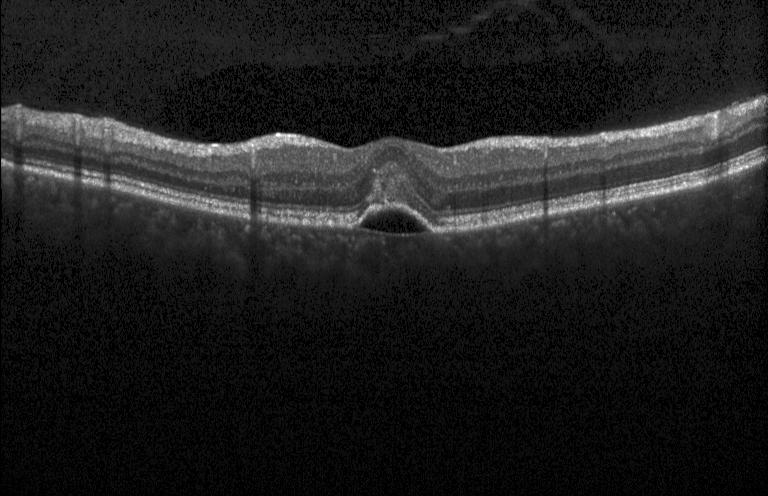

OCT B-scan
Impression: a choroidal neovascular membrane.